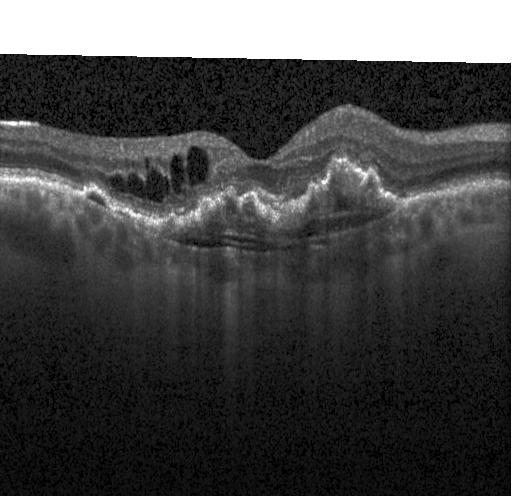

Macular scan. Retinal OCT B-scan
Macular OCT: a choroidal neovascular membrane.